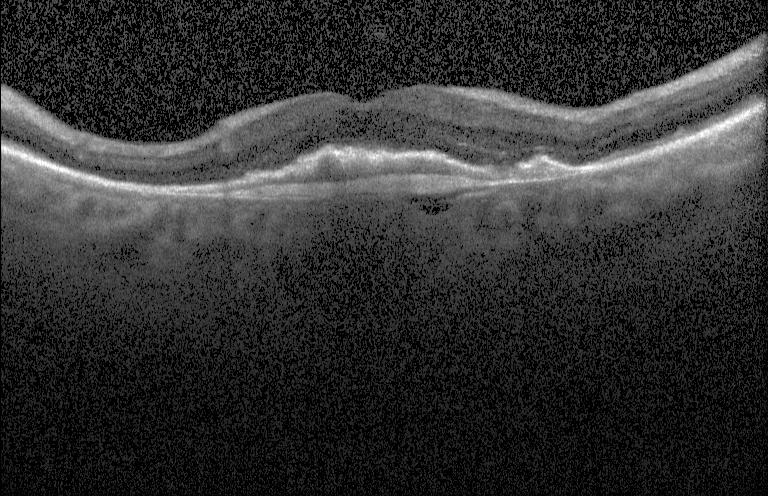

Centered on the fovea; Heidelberg Spectralis OCT system; optical coherence tomography B-scan; spectral-domain OCT — Impression: choroidal neovascularization.